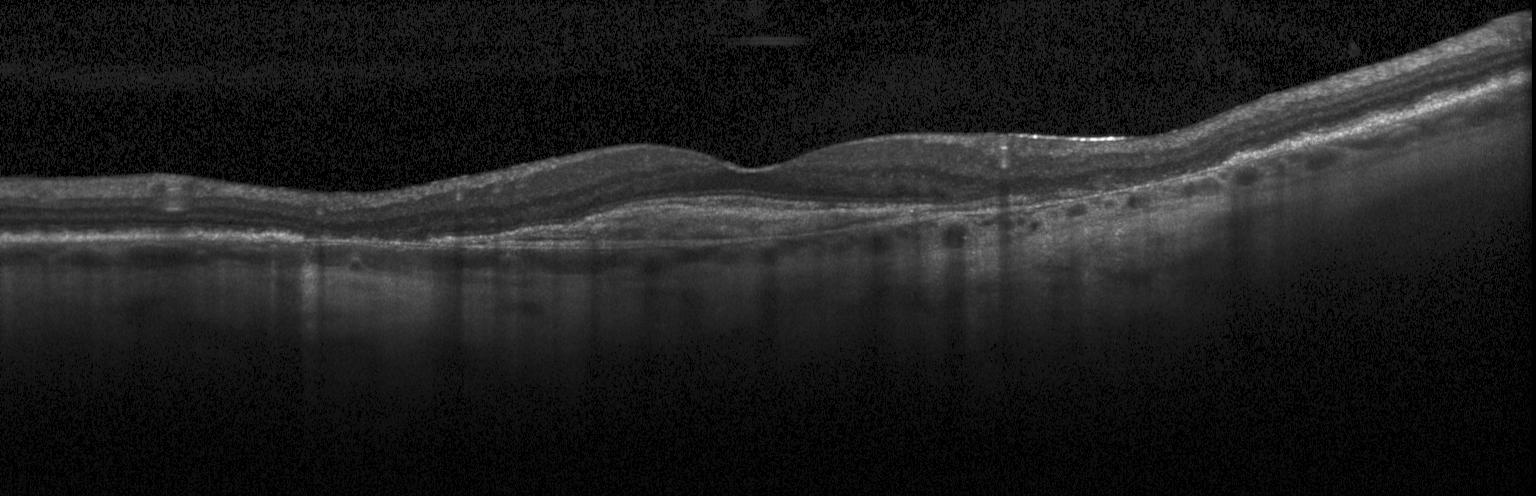 Macular OCT demonstrating choroidal neovascularization (CNV).